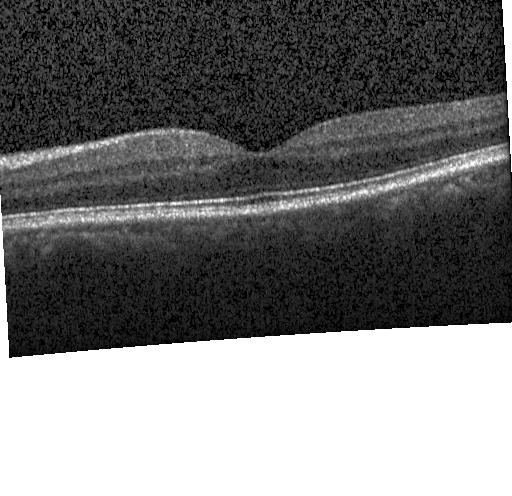

Retinal OCT B-scan · through the macula · acquired on a Heidelberg Spectralis · SD-OCT
Impression: no CNV, DME, or drusen.